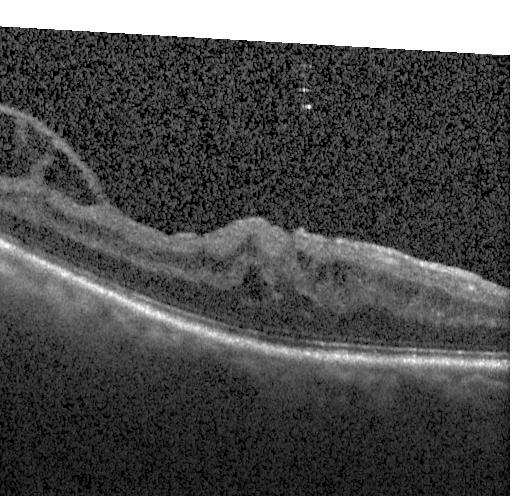
Spectral-domain OCT, centered on the fovea, Heidelberg Spectralis, retinal OCT cross-section
Finding: diabetic macular edema.